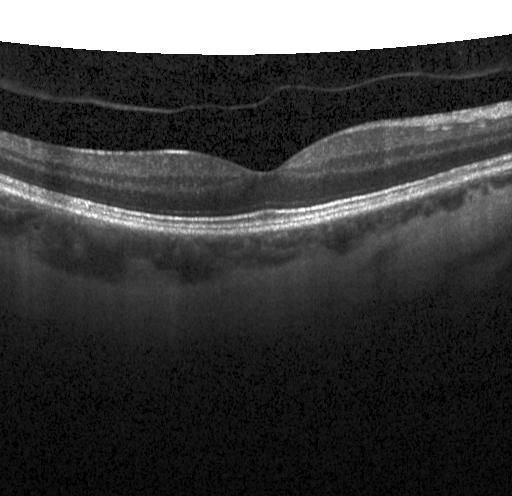 Retinal OCT B-scan. Horizontal scan through the fovea. Spectral-domain optical coherence tomography.
Finding: no evidence of CNV, DME, or drusen.